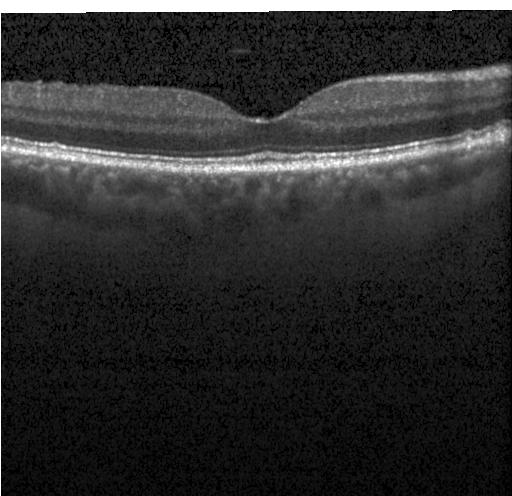 No evidence of choroidal neovascularization, diabetic macular edema, or drusen.